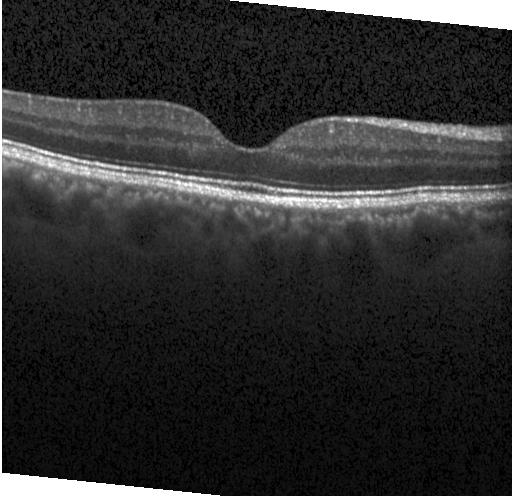

Retinal OCT cross-section — The scan shows no CNV, DME, or drusen.